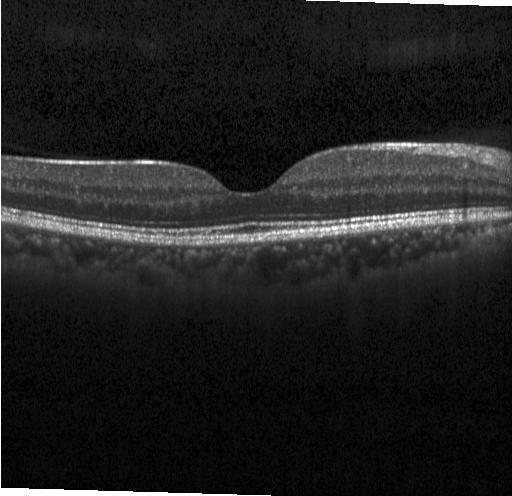 OCT line scan — Dx: no choroidal neovascularization, diabetic macular edema, or drusen.